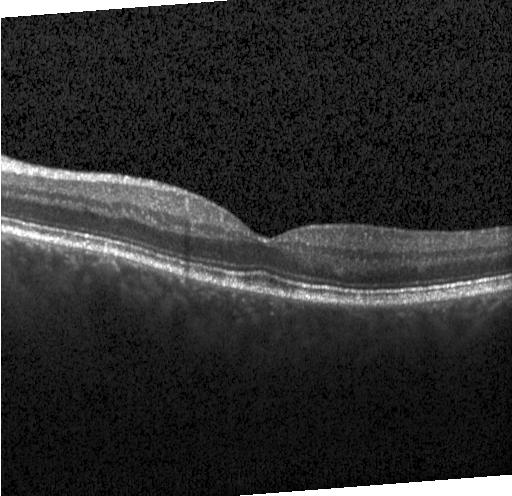
This B-scan demonstrates no choroidal neovascularization, diabetic macular edema, or drusen.